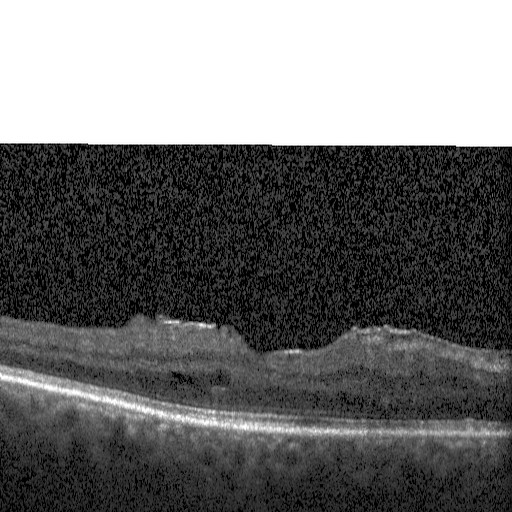

OCT scan showing diabetic macular edema.